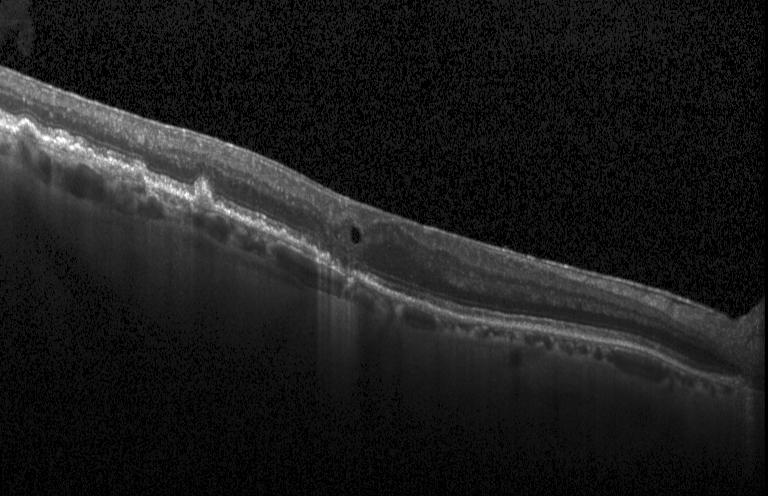
Retinal OCT cross-section.
Finding: a choroidal neovascular membrane.